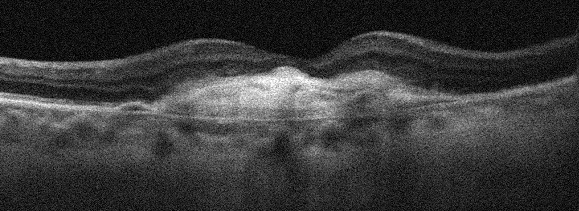
Retinal OCT B-scan, oculus sinister
Age-related macular degeneration.